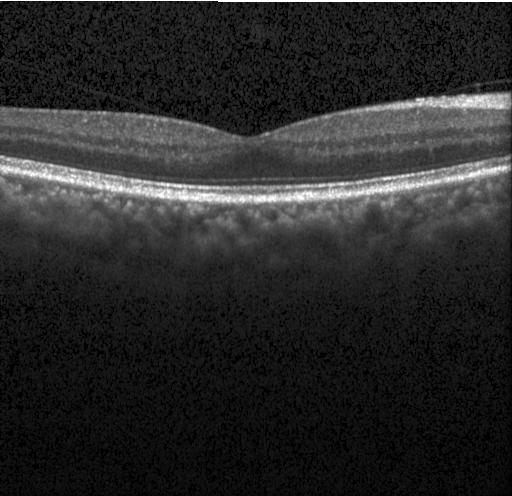 OCT B-scan showing neither choroidal neovascularization, diabetic macular edema, nor drusen.